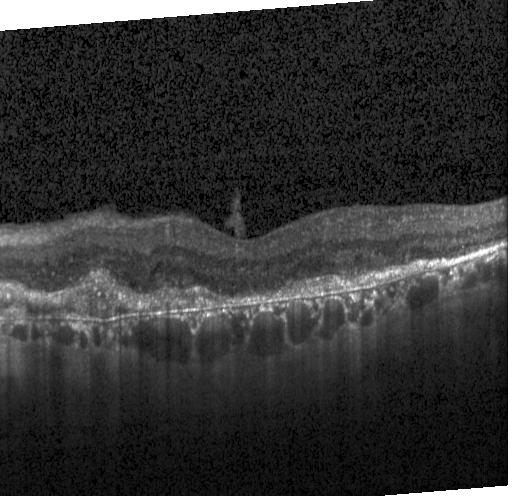
A choroidal neovascular membrane.